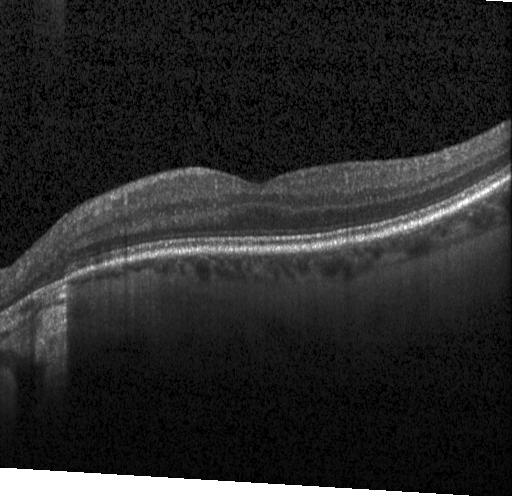

Impression: no choroidal neovascularization, diabetic macular edema, or drusen.